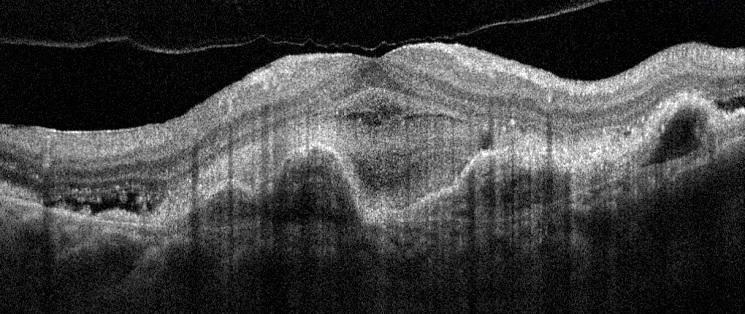

This B-scan demonstrates AMD.